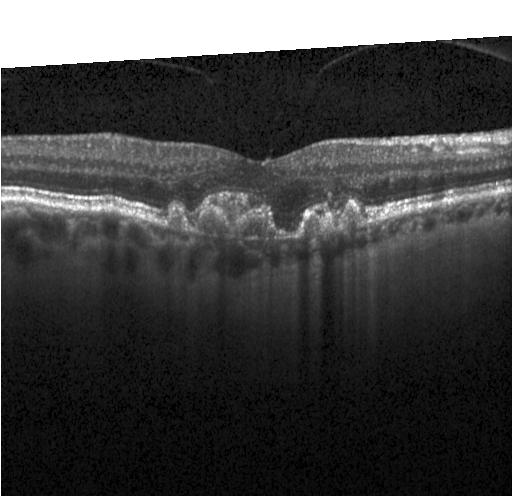 Retinal OCT cross-section.
Diagnosis: choroidal neovascularization (CNV).